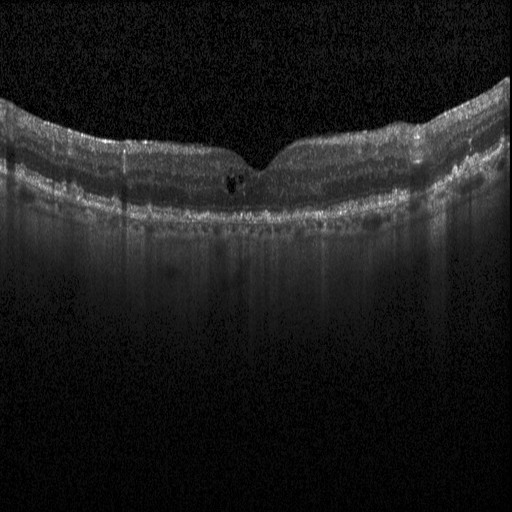
OCT finding: diabetic macular edema (DME).